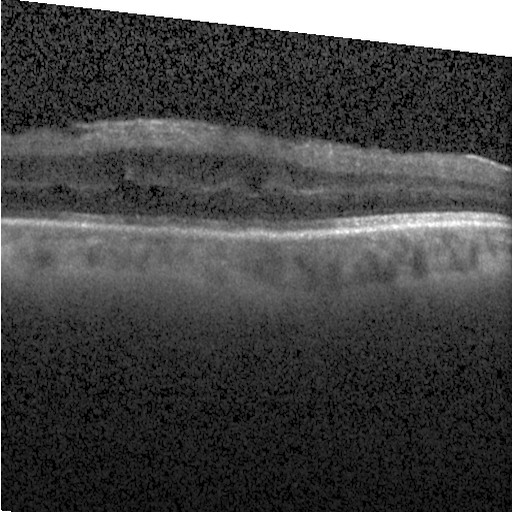
OCT B-scan — Macular OCT: diabetic macular edema.